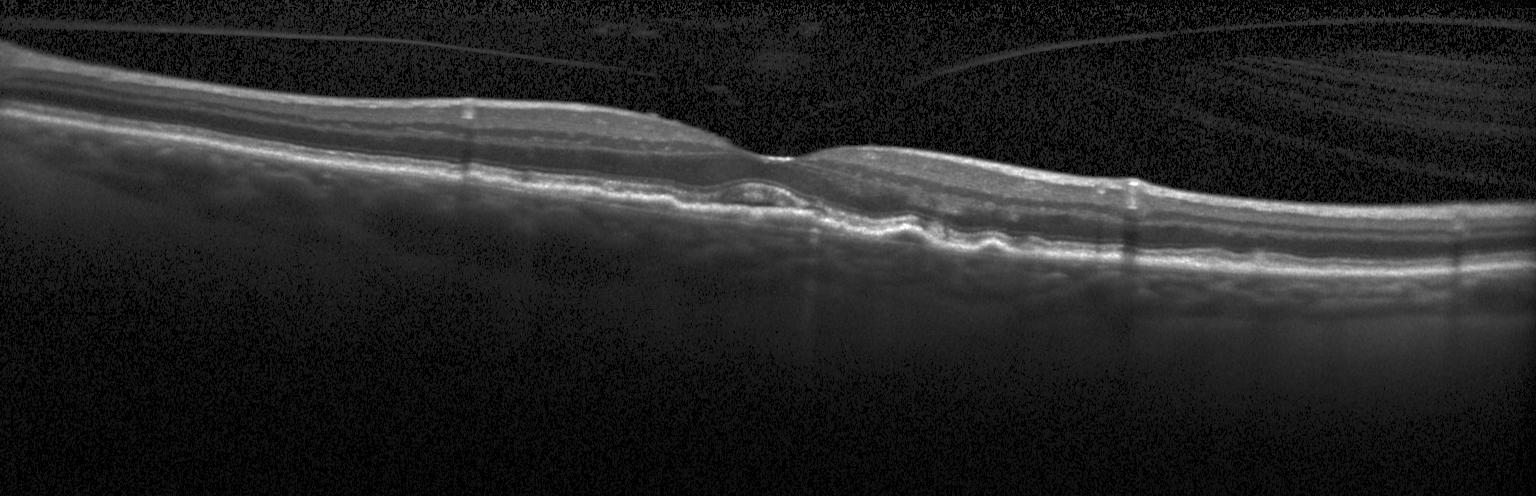 Optical coherence tomography scan; spectral-domain optical coherence tomography; horizontal scan through the fovea. Impression: a choroidal neovascular membrane.